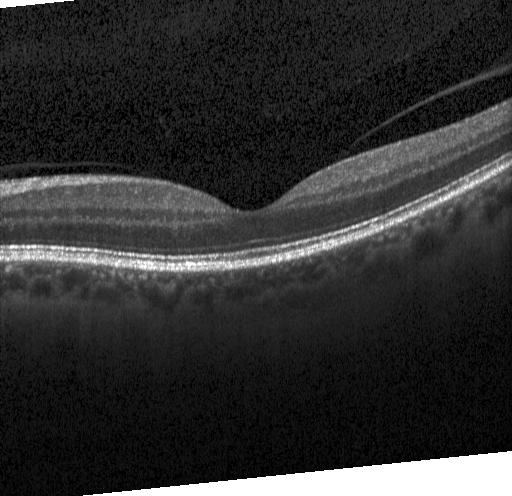
Diagnosis: no choroidal neovascularization, diabetic macular edema, or drusen.